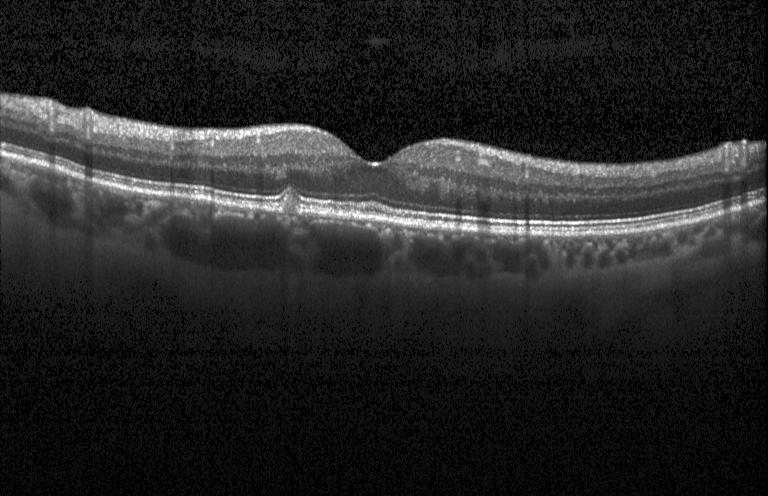
Centered on the fovea; retinal OCT cross-section; spectral-domain optical coherence tomography.
Impression: sub-RPE drusenoid deposits.